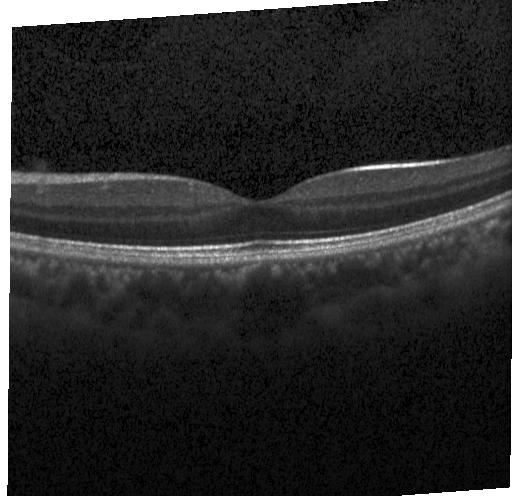
Finding: no evidence of choroidal neovascularization, diabetic macular edema, or drusen.